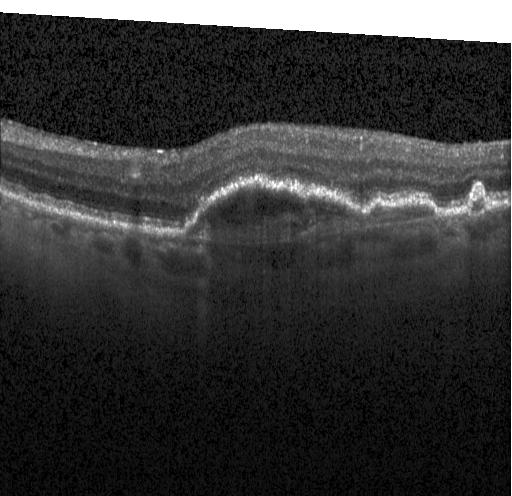 The scan shows a choroidal neovascular membrane.